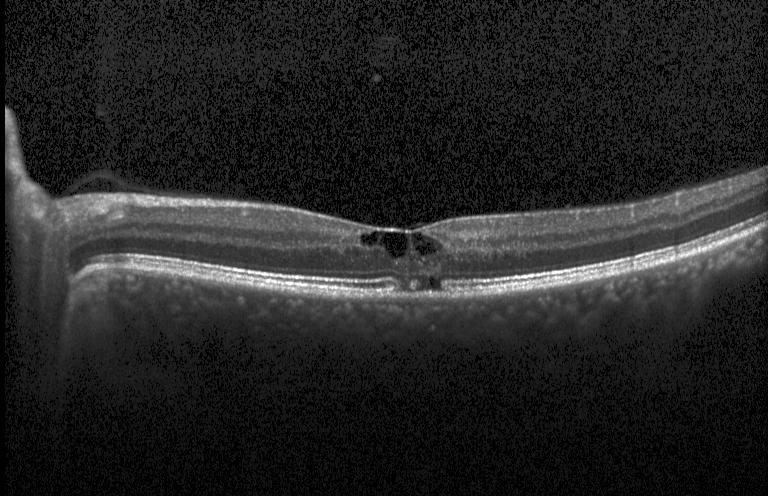
Heidelberg Spectralis. Horizontal scan through the fovea. OCT B-scan — Impression: diabetic macular edema (DME).